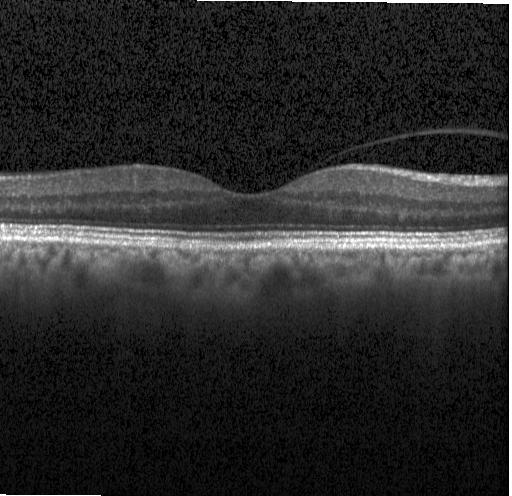

SD-OCT, retinal OCT cross-section
Assessment: neither choroidal neovascularization, diabetic macular edema, nor drusen.